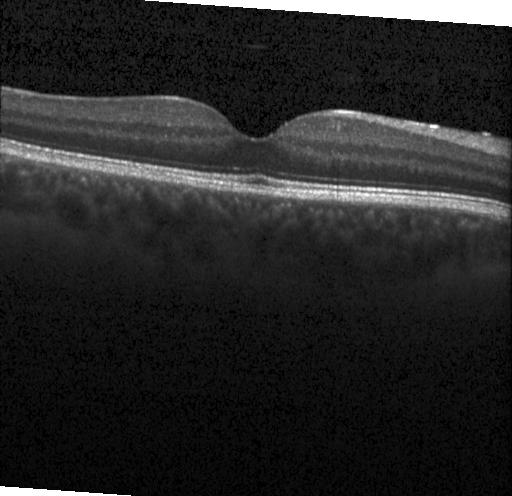 Macular OCT demonstrating no choroidal neovascularization, diabetic macular edema, or drusen.